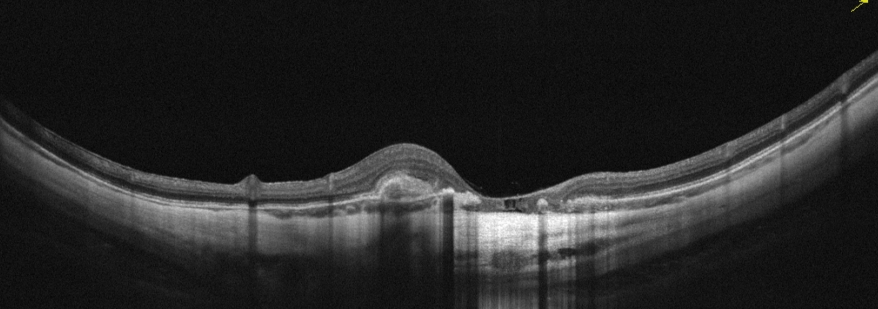 Diagnosis: AMD.